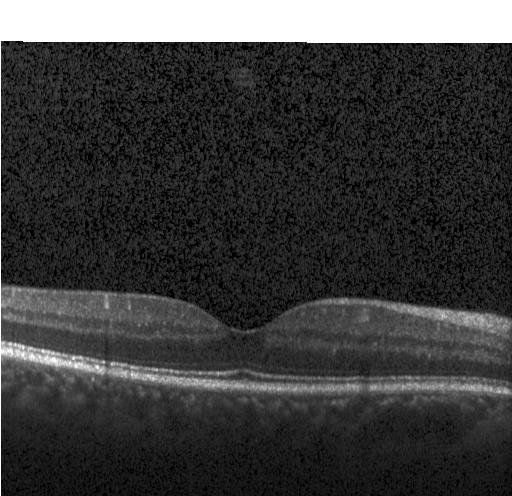

Heidelberg Spectralis OCT system · spectral-domain optical coherence tomography · horizontal scan through the fovea · optical coherence tomography scan
The scan shows no evidence of CNV, DME, or drusen.